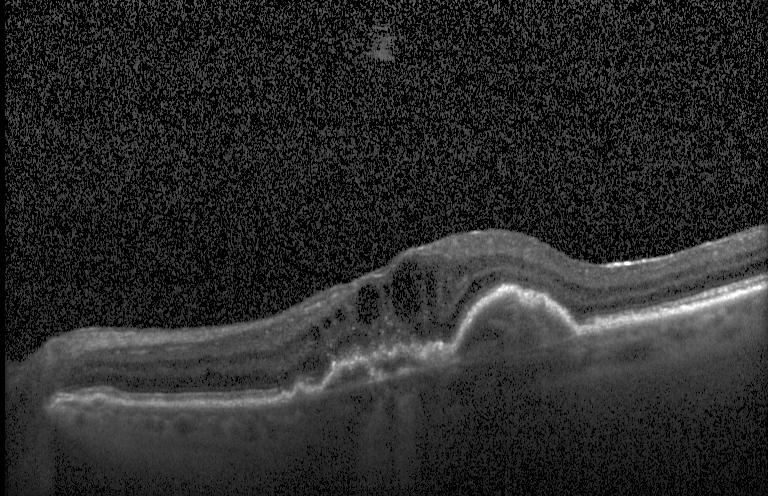

Optical coherence tomography B-scan, SD-OCT, Heidelberg Spectralis.
Impression: CNV.